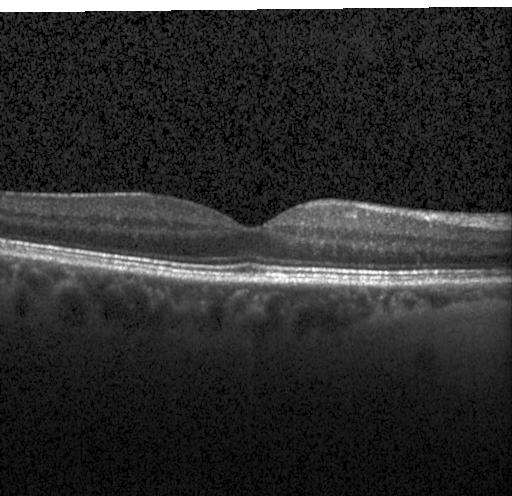 OCT line scan. SD-OCT. Impression: no CNV, DME, or drusen.